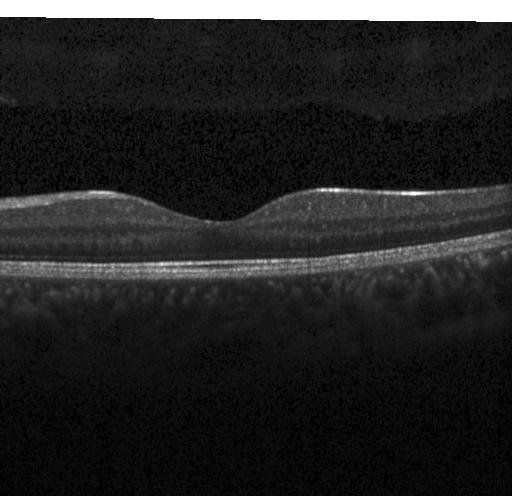
SD-OCT; OCT B-scan.
OCT finding: no CNV, no DME, and no drusen.